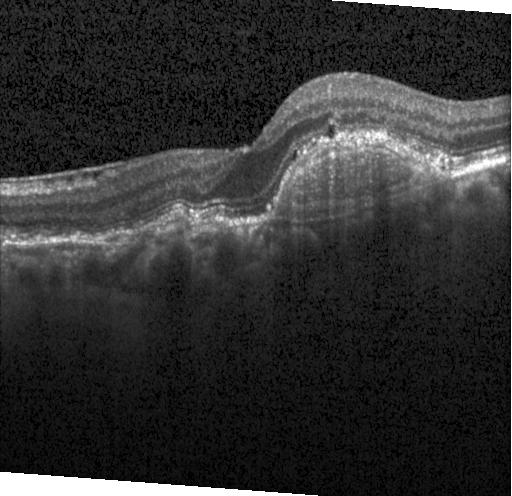

SD-OCT · OCT B-scan. Diagnosis: choroidal neovascularization.